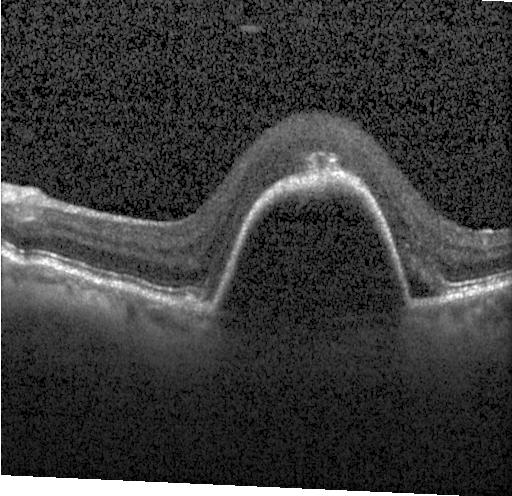 Instrument: Heidelberg Spectralis, horizontal scan through the fovea, optical coherence tomography B-scan, spectral-domain OCT.
OCT finding: CNV.